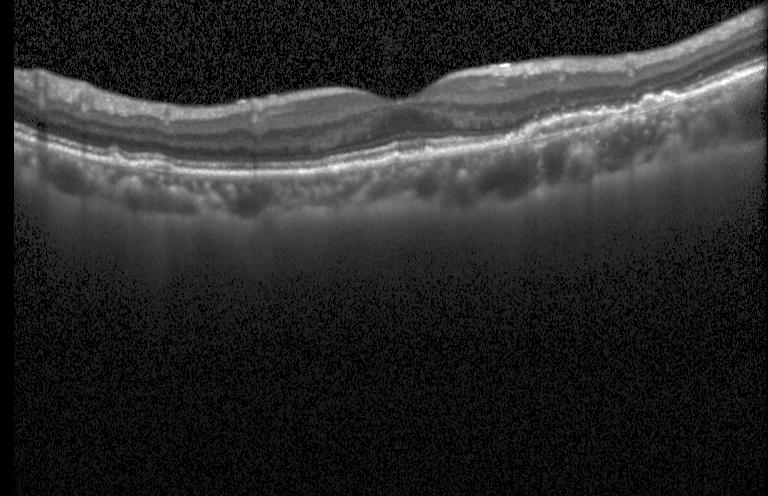

Spectral-domain OCT B-scan: a choroidal neovascular membrane.